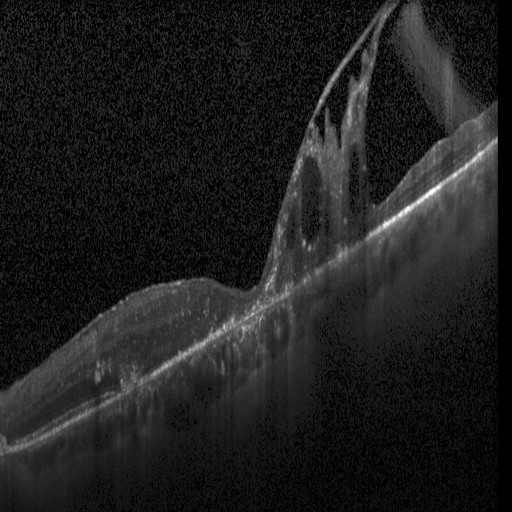

Diagnosis: diabetic macular edema.